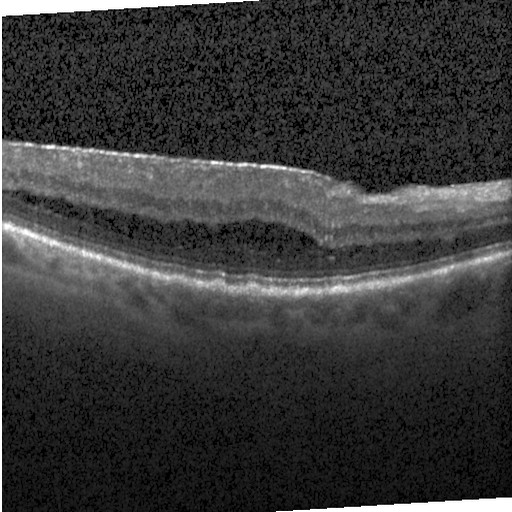
OCT B-scan showing DME.